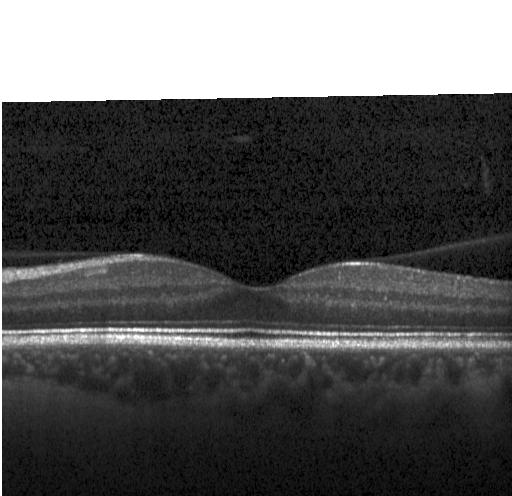 OCT line scan — OCT finding: no choroidal neovascularization, no diabetic macular edema, and no drusen.